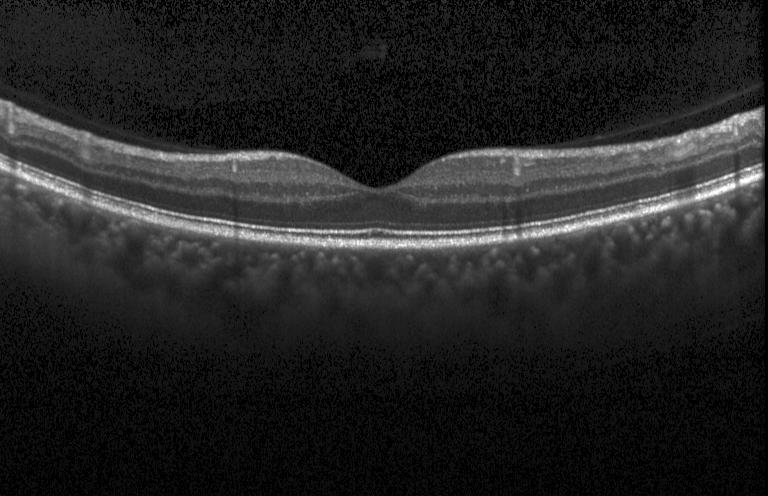

The scan shows neither CNV, DME, nor drusen.